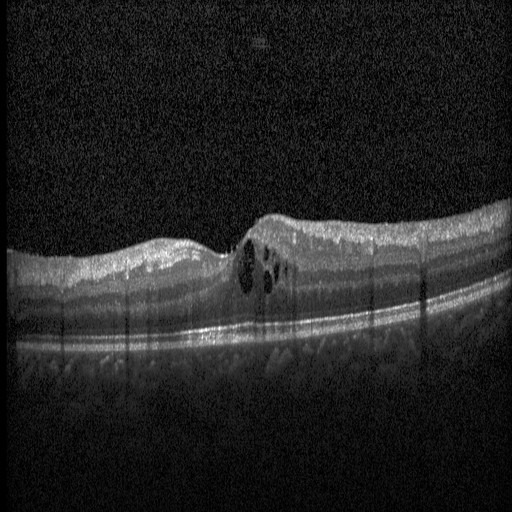
Optical coherence tomography scan. Through the macula — Finding: diabetic macular edema (DME).